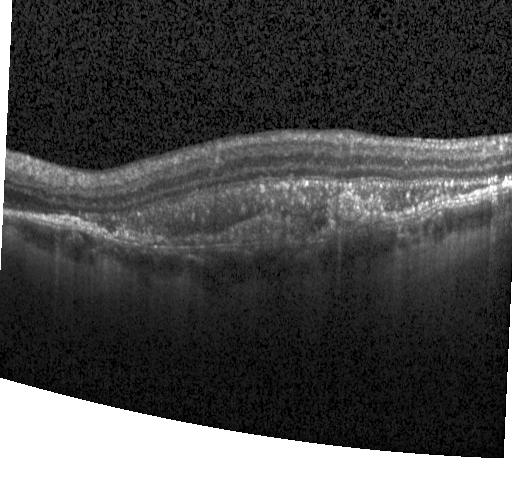
Retinal OCT cross-section. SD-OCT. Instrument: Heidelberg Spectralis — CNV.